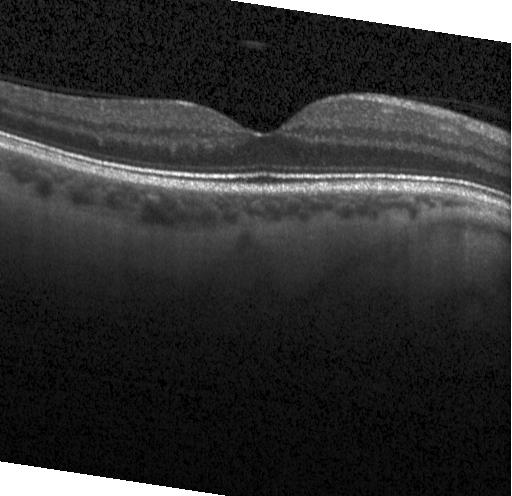

Macular scan · Heidelberg Spectralis · optical coherence tomography B-scan · spectral-domain OCT — Diagnosis: no choroidal neovascularization, diabetic macular edema, or drusen.